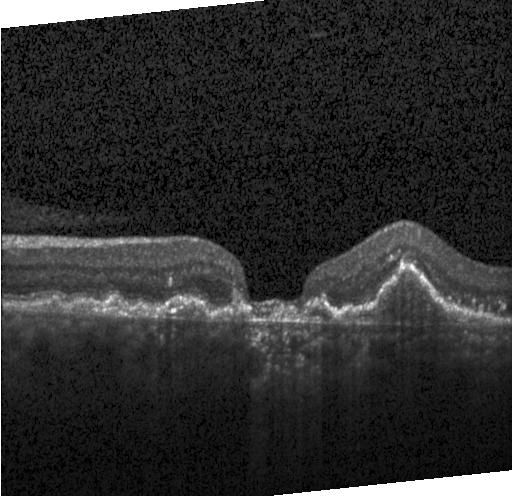

Choroidal neovascularization.